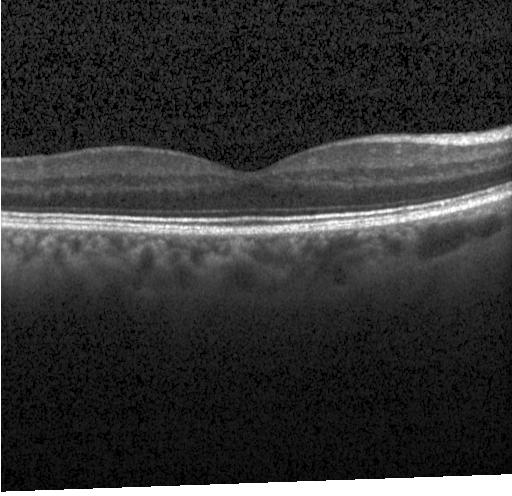 Through the macula, OCT line scan, SD-OCT, Heidelberg Spectralis OCT system.
This B-scan demonstrates neither choroidal neovascularization, diabetic macular edema, nor drusen.